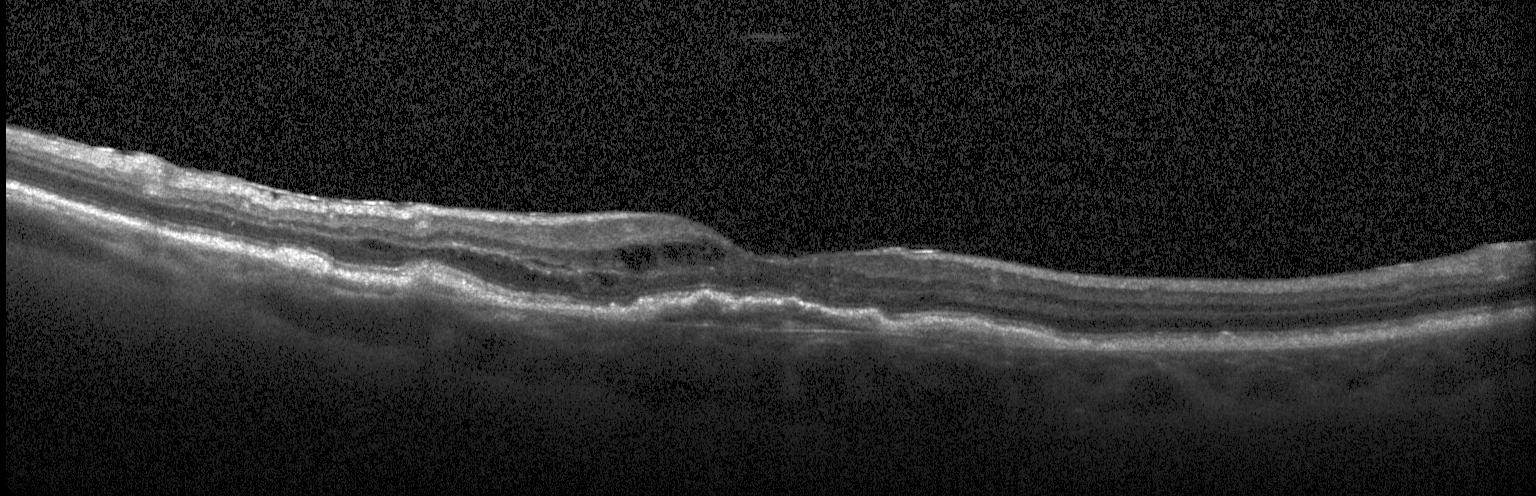 Impression: a choroidal neovascular membrane.